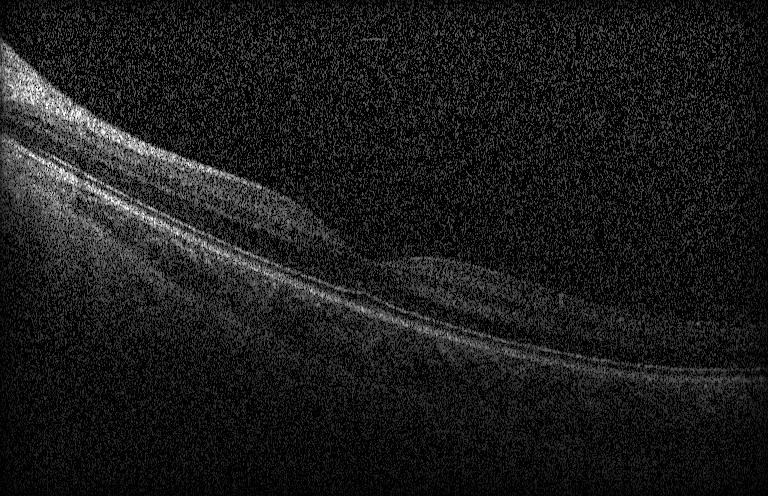

Retinal OCT cross-section.
This B-scan demonstrates no CNV, no DME, and no drusen.